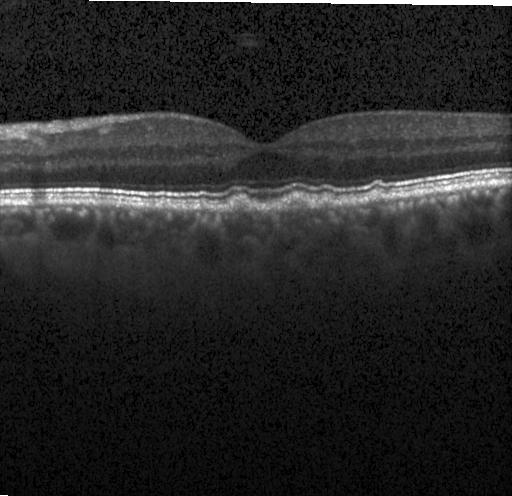
Spectral-domain OCT B-scan: sub-RPE drusenoid deposits.